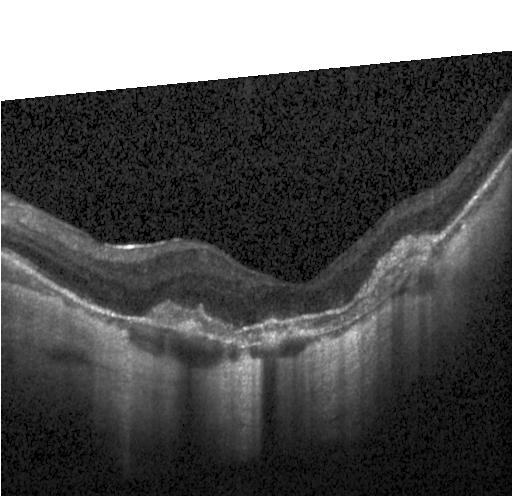

Spectral-domain optical coherence tomography; Heidelberg Spectralis OCT system; centered on the fovea; OCT B-scan.
Assessment: choroidal neovascularization.